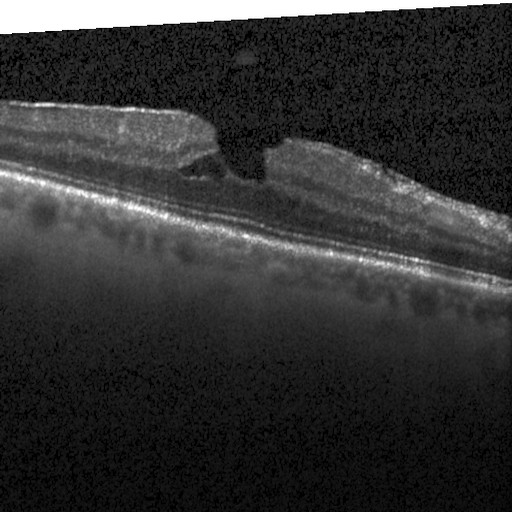

Finding: diabetic macular edema.